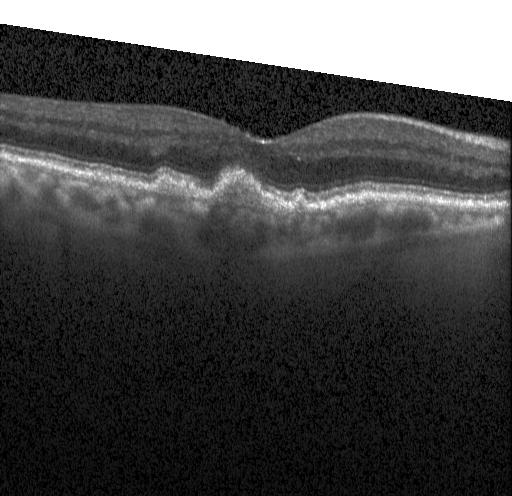

The scan shows drusen.